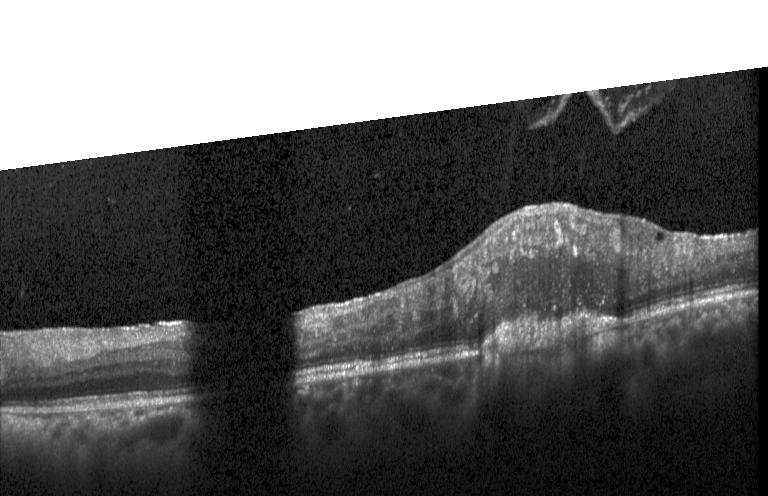 SD-OCT, optical coherence tomography B-scan
Finding: CNV.